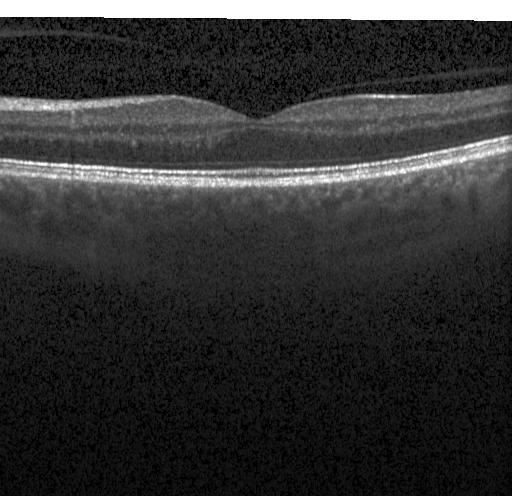
Fovea-centered · spectral-domain optical coherence tomography · OCT line scan
This B-scan demonstrates no choroidal neovascularization, no diabetic macular edema, and no drusen.